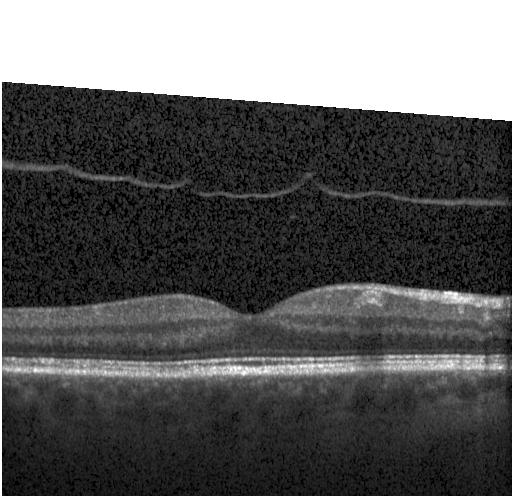 OCT B-scan. Spectral-domain OCT. Centered on the fovea. Finding: no evidence of CNV, DME, or drusen.